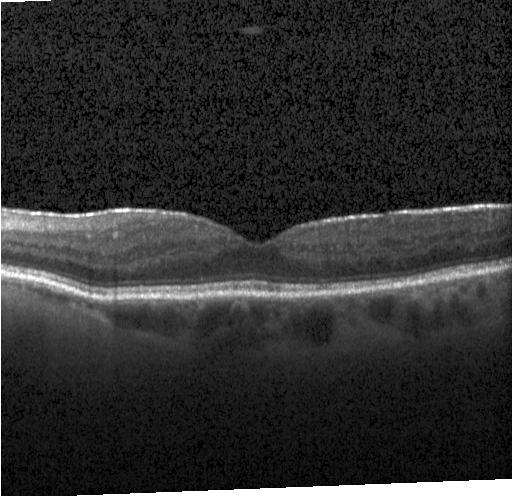

The scan shows no CNV, DME, or drusen.